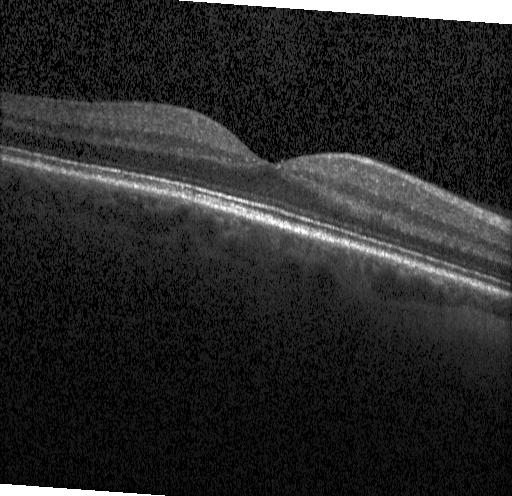 OCT B-scan
The scan shows no CNV, DME, or drusen.